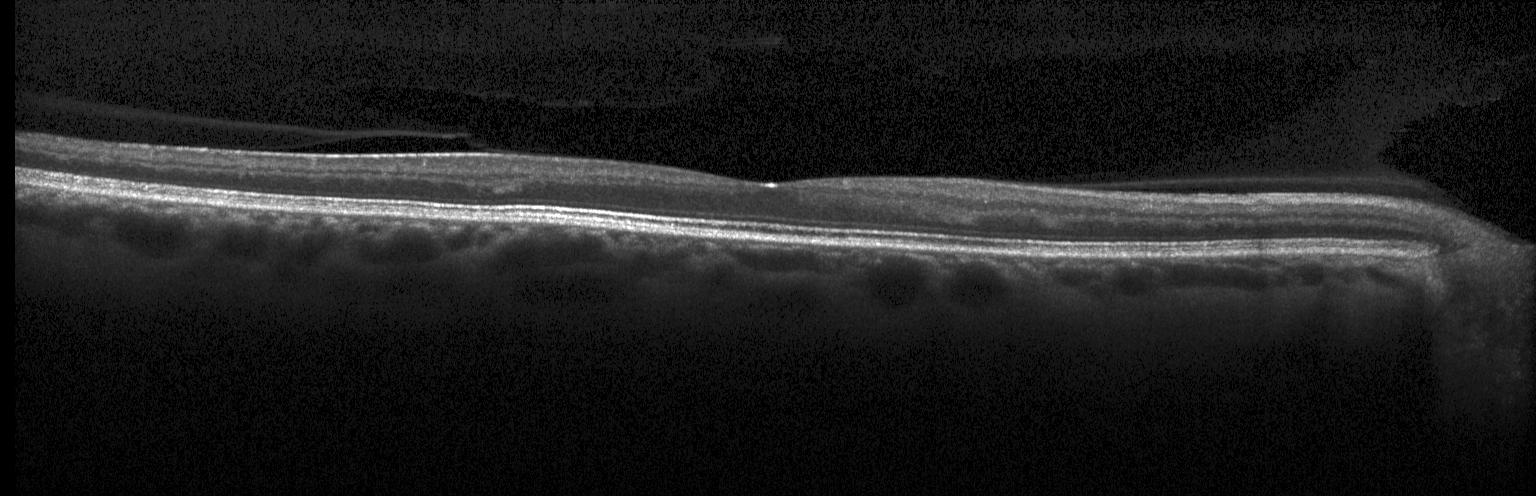

Through the macula, retinal OCT B-scan.
The scan shows no choroidal neovascularization, diabetic macular edema, or drusen.